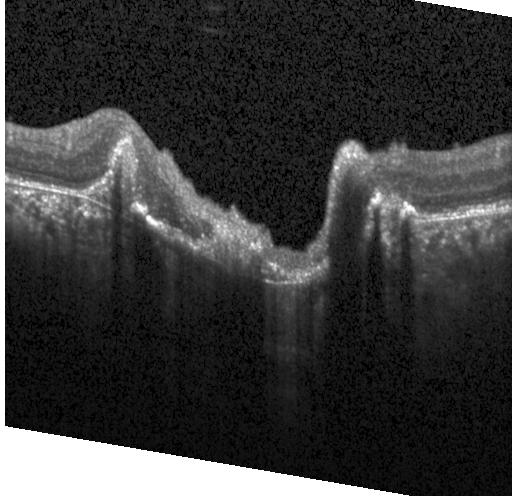

A choroidal neovascular membrane.